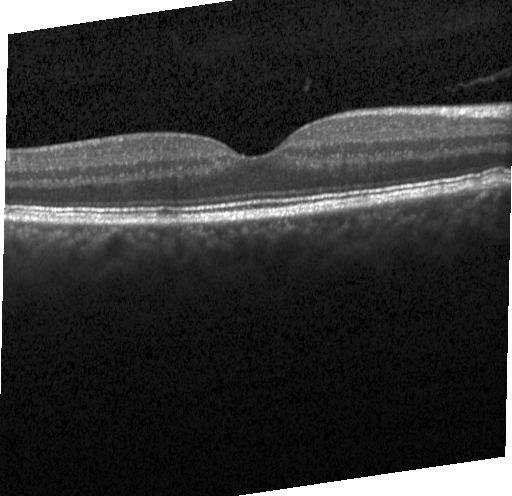 Heidelberg Spectralis; centered on the fovea; optical coherence tomography B-scan; spectral-domain OCT. Macular OCT: neither CNV, DME, nor drusen.